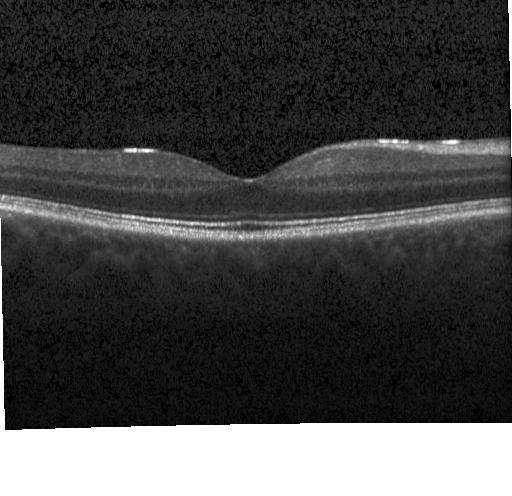

Neither choroidal neovascularization, diabetic macular edema, nor drusen.